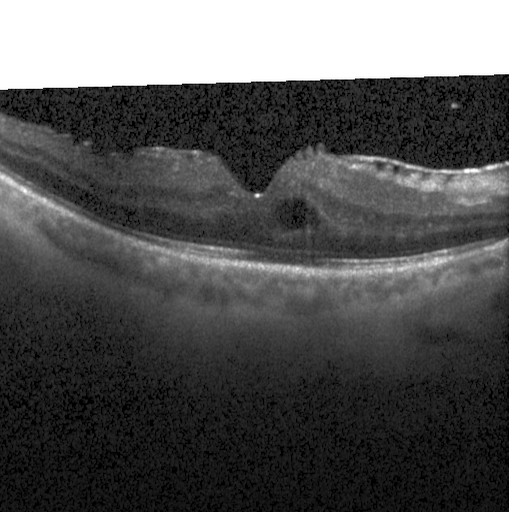
Retinal OCT cross-section showing DME.